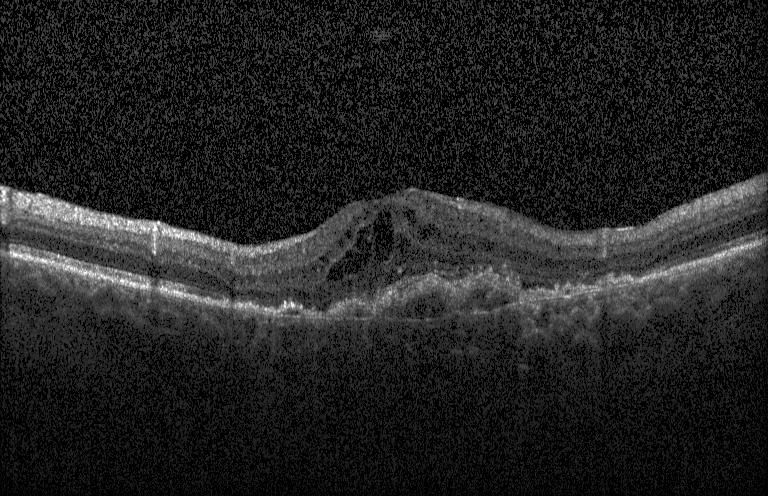 Heidelberg Spectralis; spectral-domain OCT; horizontal scan through the fovea; optical coherence tomography B-scan.
Diagnosis: CNV.